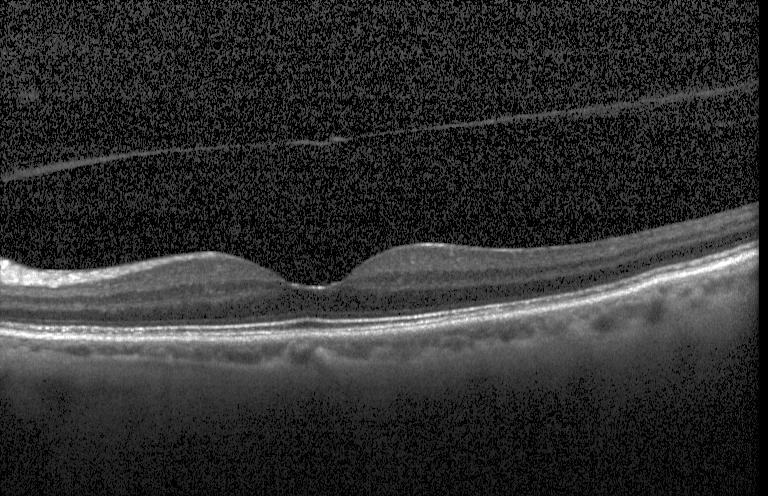 SD-OCT. Optical coherence tomography B-scan. Horizontal scan through the fovea. Diagnosis: no evidence of CNV, DME, or drusen.